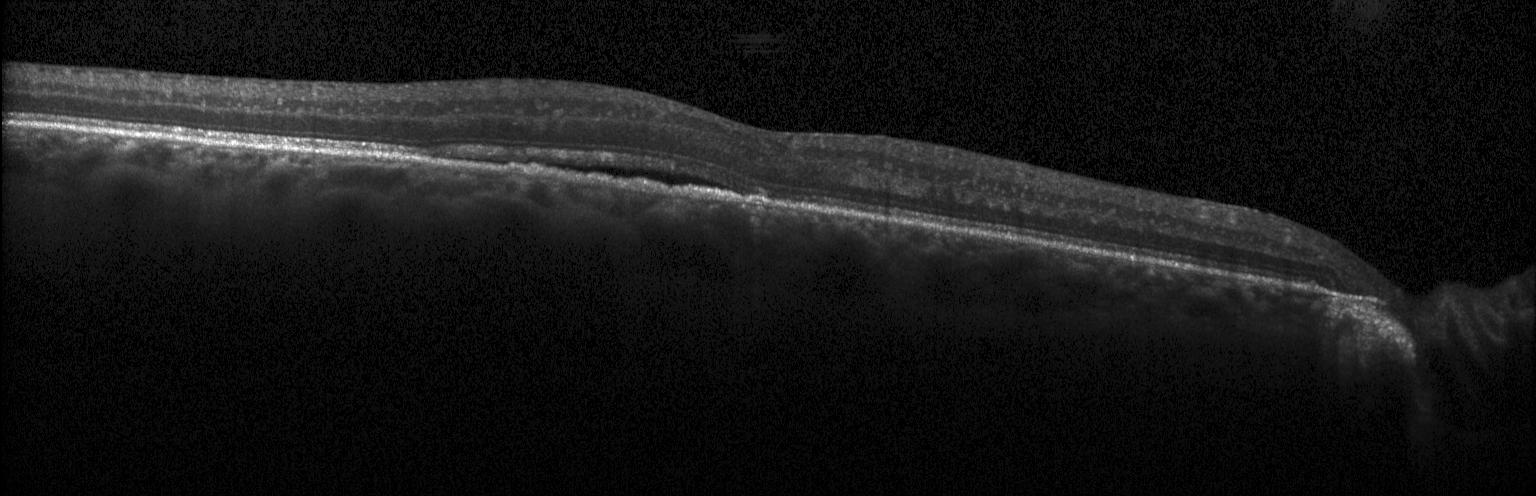

Spectral-domain OCT, retinal OCT B-scan, Heidelberg Spectralis OCT system
Finding: a choroidal neovascular membrane.